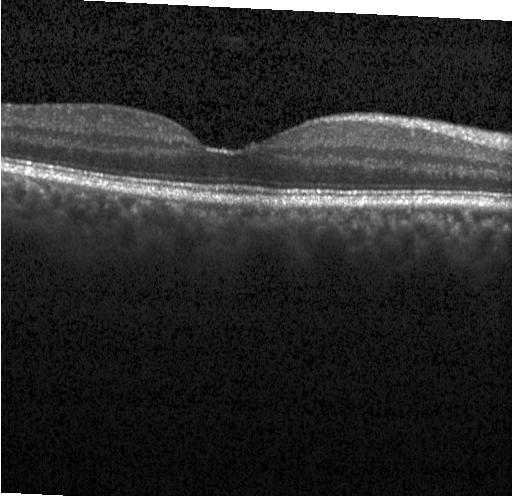
The scan shows no choroidal neovascularization, diabetic macular edema, or drusen.